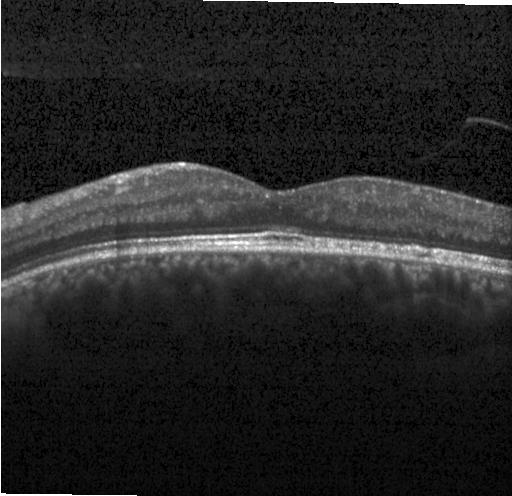
OCT line scan — Finding: no CNV, DME, or drusen.